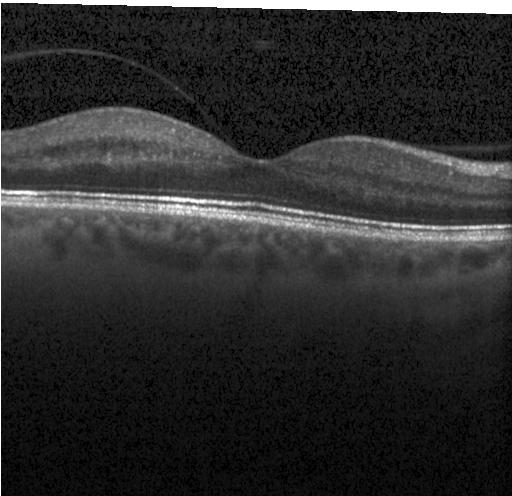

Spectral-domain OCT B-scan: diabetic macular edema (DME).